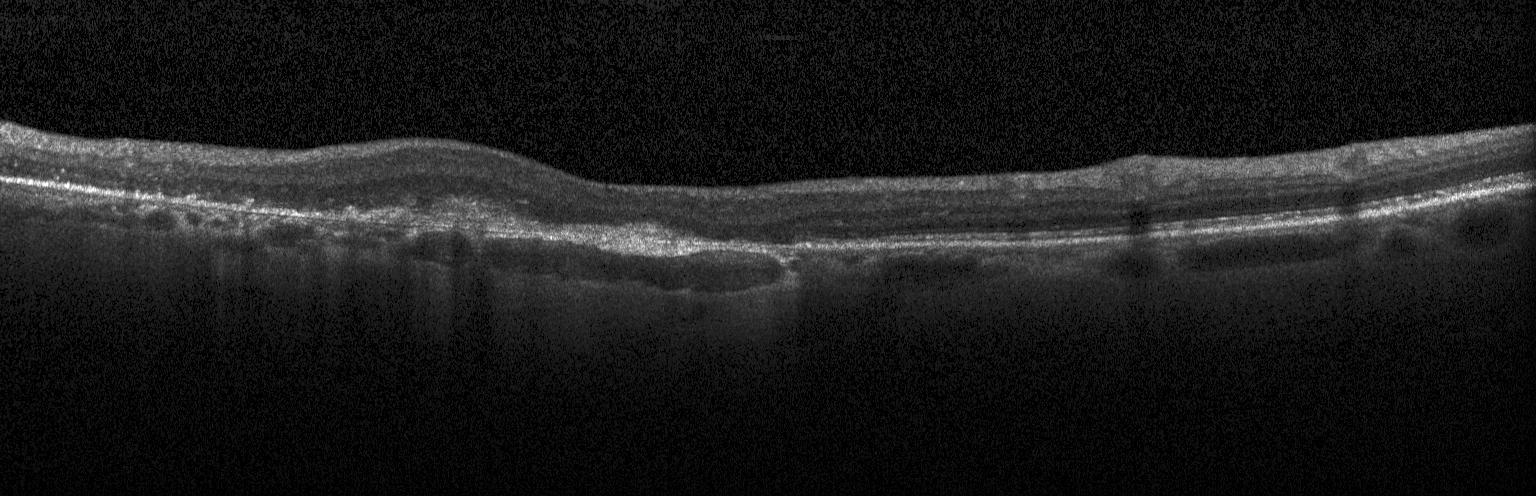 OCT line scan — A choroidal neovascular membrane.